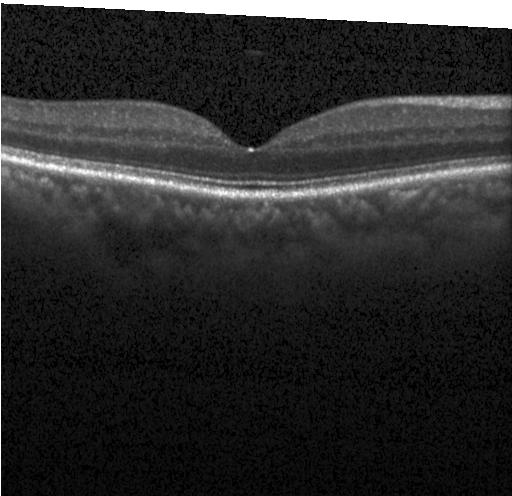
Spectral-domain OCT B-scan: no choroidal neovascularization, diabetic macular edema, or drusen.